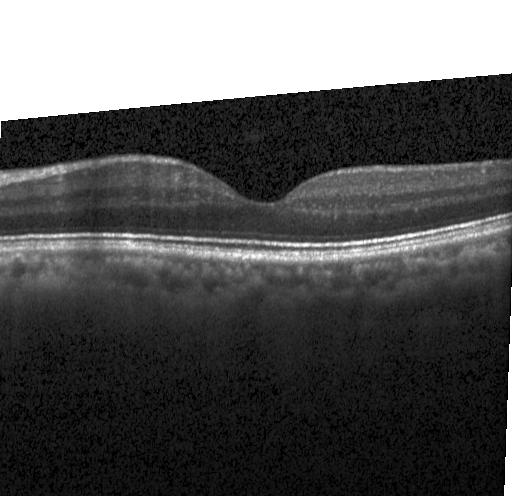 SD-OCT, optical coherence tomography scan, instrument: Heidelberg Spectralis — Dx: neither choroidal neovascularization, diabetic macular edema, nor drusen.